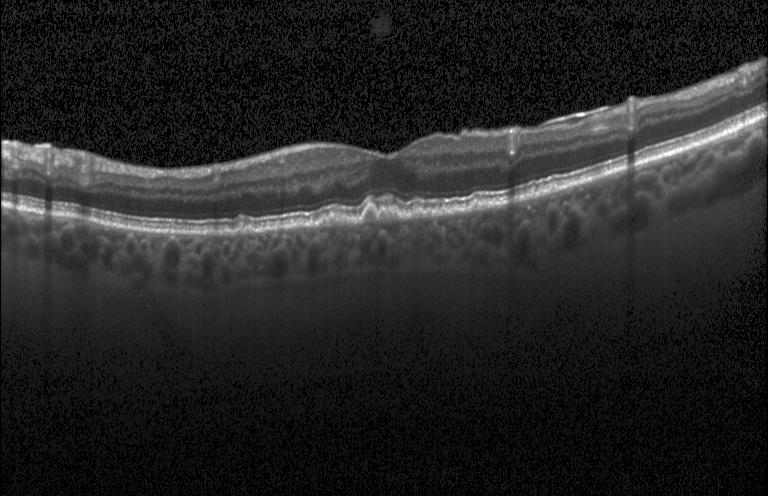 Spectral-domain optical coherence tomography. Optical coherence tomography B-scan. Heidelberg Spectralis.
Diagnosis: drusen.